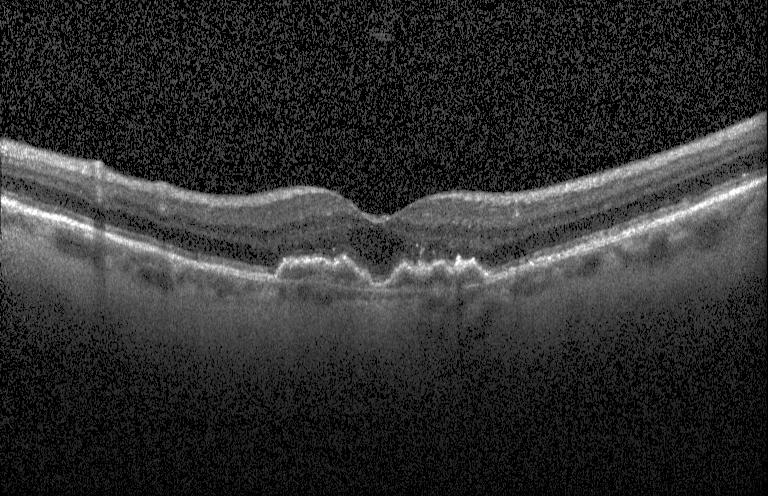
Optical coherence tomography scan
Impression: choroidal neovascularization (CNV).